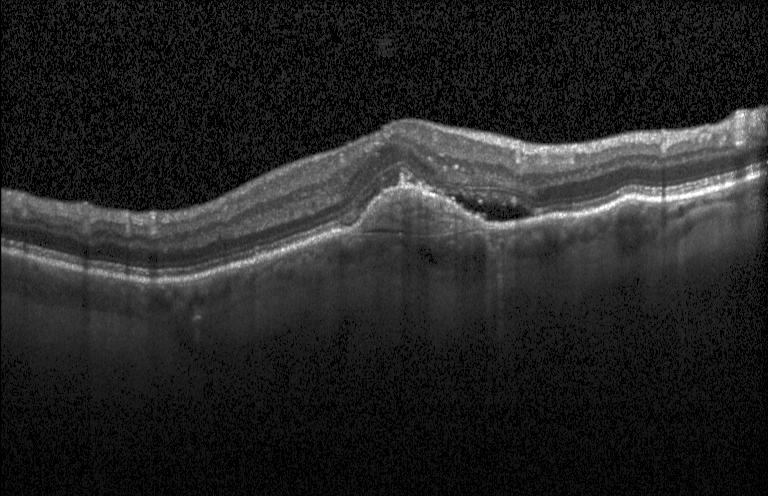

OCT B-scan showing choroidal neovascularization (CNV).